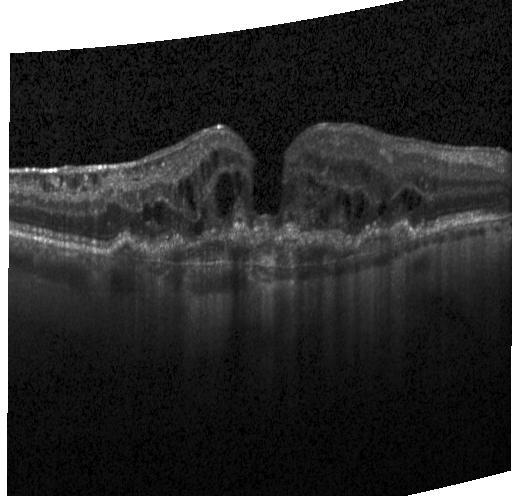

Optical coherence tomography B-scan
Diagnosis: a choroidal neovascular membrane.